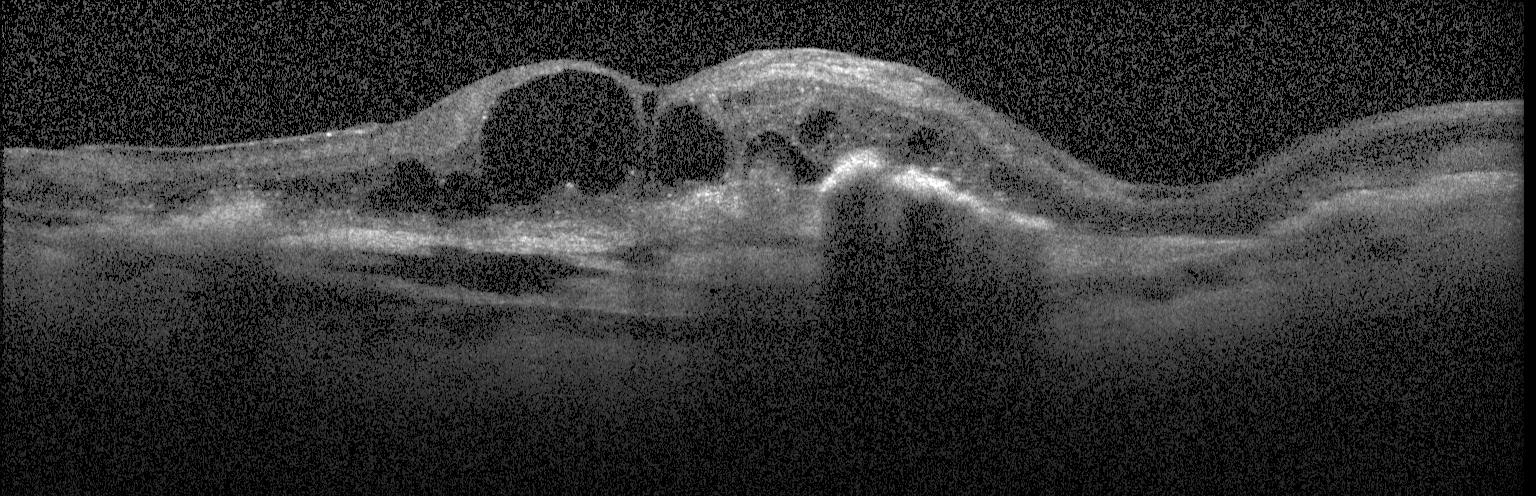 Acquired on a Heidelberg Spectralis · spectral-domain optical coherence tomography · OCT B-scan — Diagnosis: a choroidal neovascular membrane.